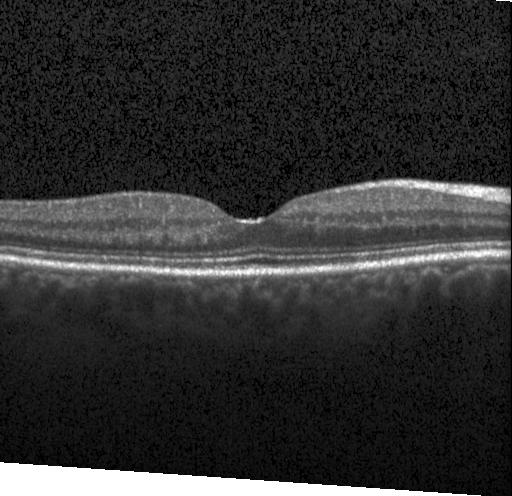

Retinal OCT B-scan. Neither CNV, DME, nor drusen.